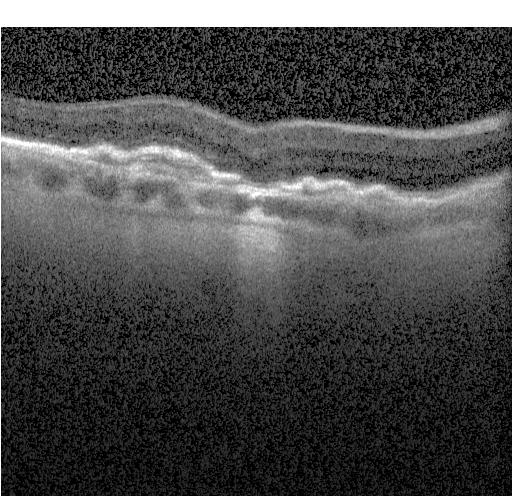
Centered on the fovea; OCT line scan; Heidelberg Spectralis OCT system — Diagnosis: a choroidal neovascular membrane.